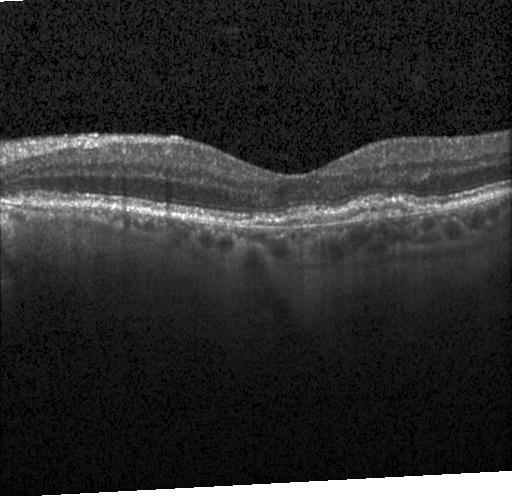
Spectral-domain OCT · through the macula · optical coherence tomography B-scan
This B-scan demonstrates choroidal neovascularization.